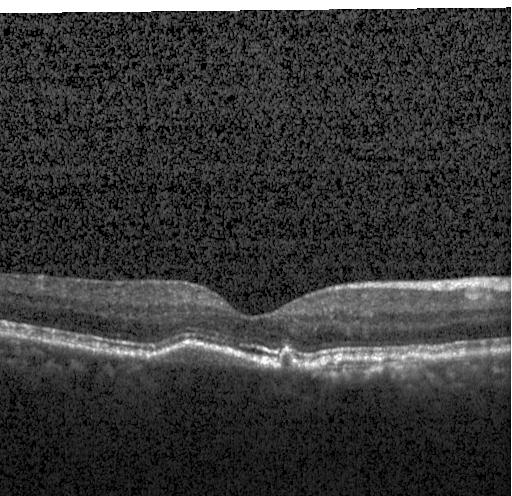 Fovea-centered · SD-OCT · retinal OCT cross-section — Macular OCT: drusen.